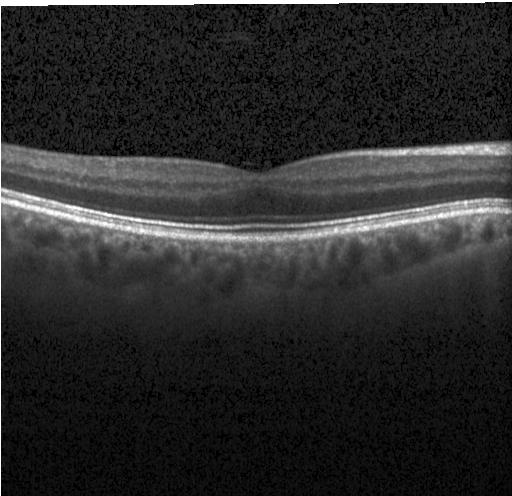 Spectral-domain OCT B-scan: no choroidal neovascularization, diabetic macular edema, or drusen.